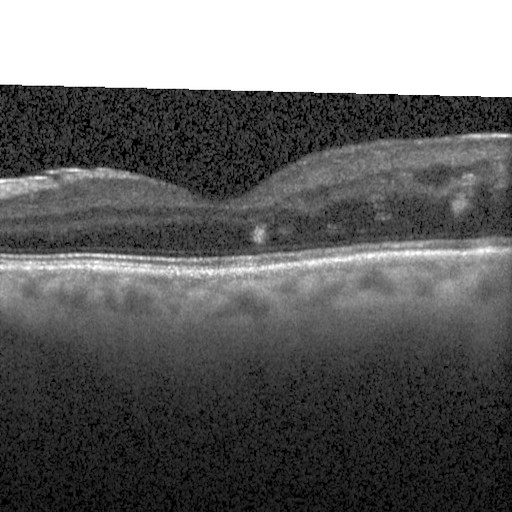 Finding: diabetic macular edema.